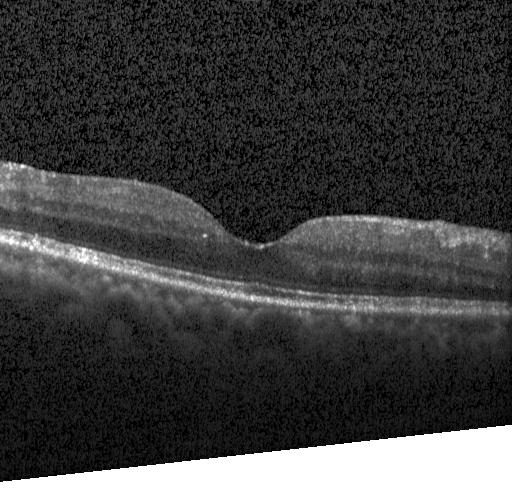 This B-scan demonstrates no CNV, DME, or drusen.